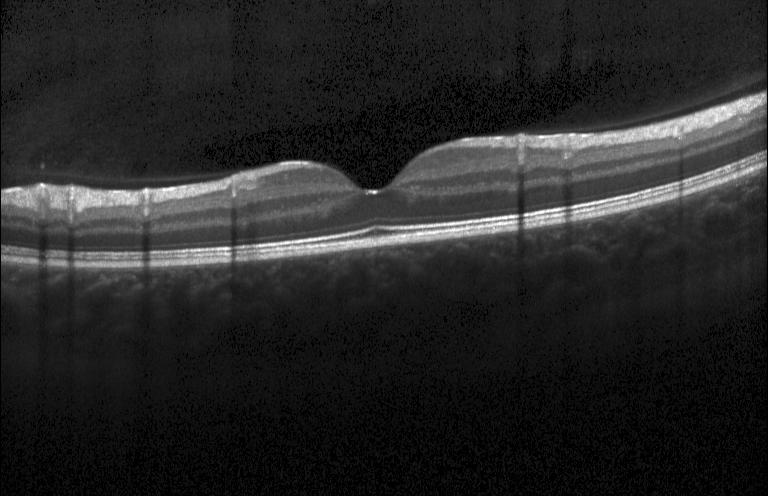
OCT B-scan. Instrument: Heidelberg Spectralis. SD-OCT. Macular scan. Impression: no CNV, DME, or drusen.